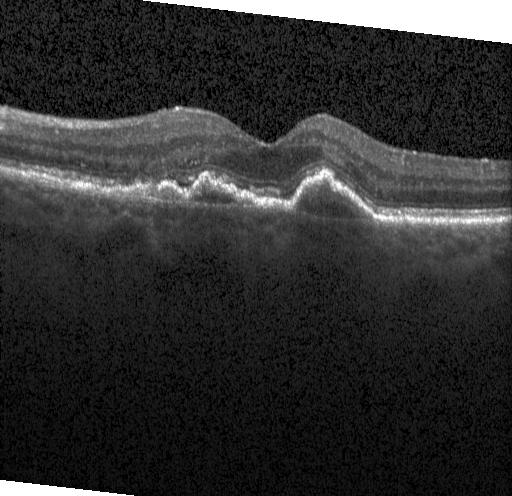
Optical coherence tomography B-scan; acquired on a Heidelberg Spectralis — Impression: choroidal neovascularization (CNV).